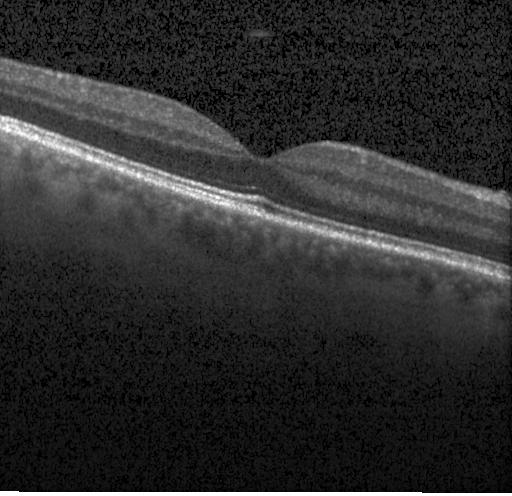
SD-OCT · OCT B-scan · Heidelberg Spectralis OCT system · macular scan. No CNV, DME, or drusen.